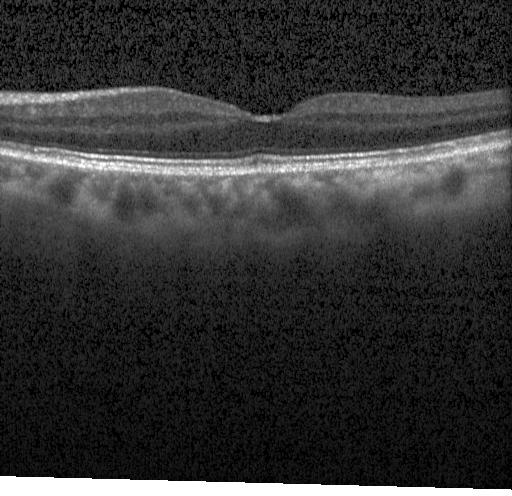

OCT line scan. This B-scan demonstrates neither CNV, DME, nor drusen.